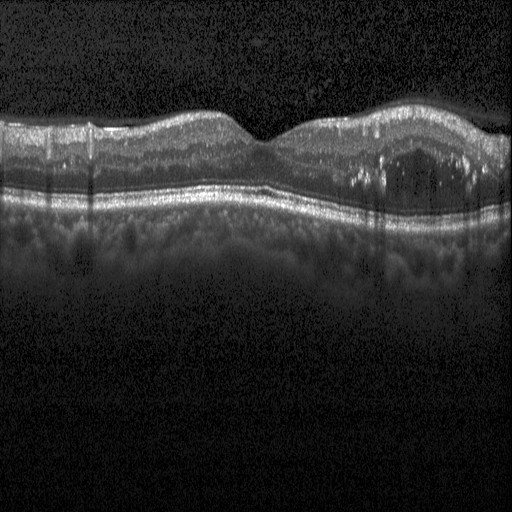 OCT scan showing DME.